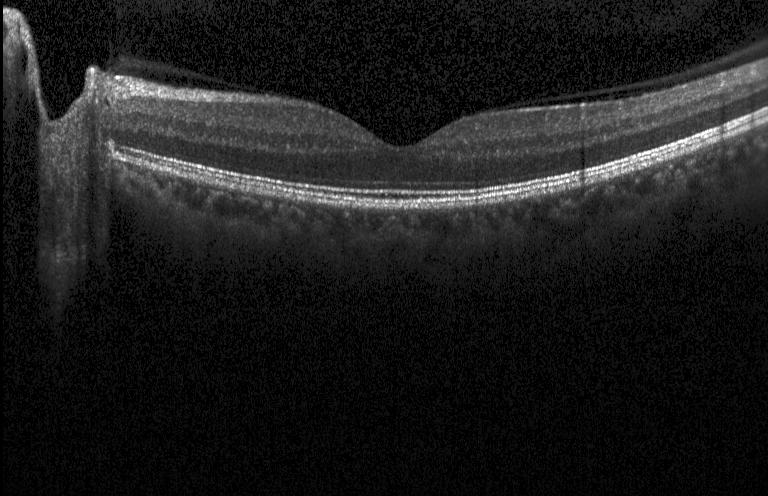

Assessment: neither choroidal neovascularization, diabetic macular edema, nor drusen.